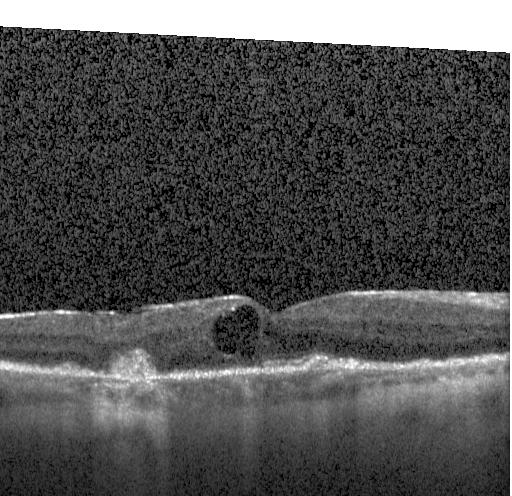

OCT line scan. Spectral-domain optical coherence tomography.
Assessment: a choroidal neovascular membrane.